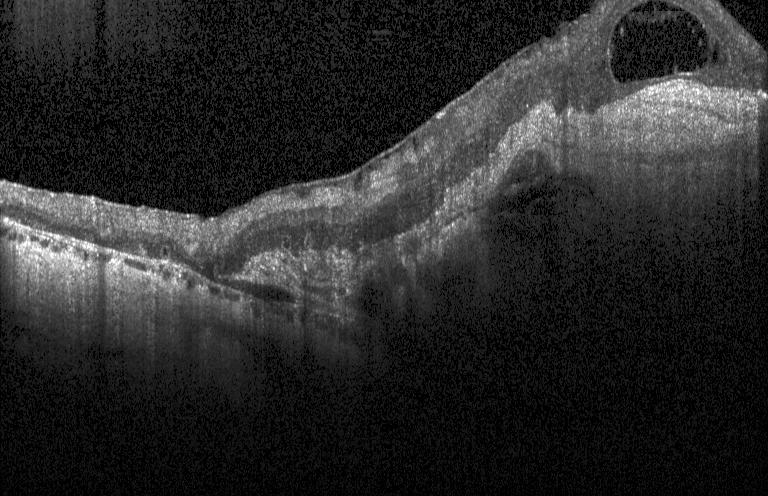
OCT line scan — Finding: choroidal neovascularization.